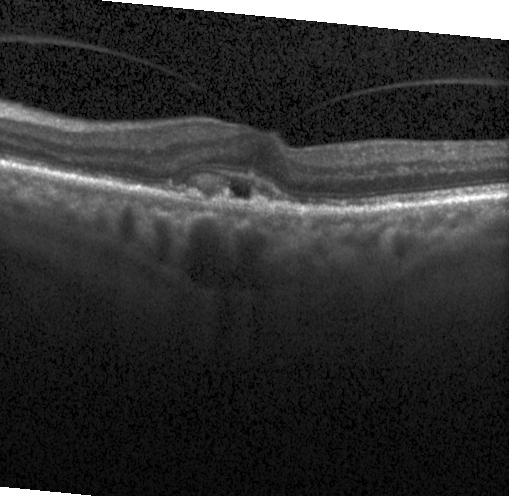
This B-scan demonstrates a choroidal neovascular membrane.